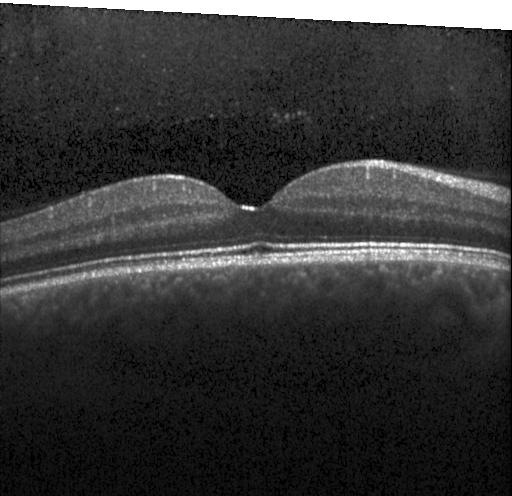

Instrument: Heidelberg Spectralis; OCT line scan; SD-OCT; through the macula — Macular OCT: neither choroidal neovascularization, diabetic macular edema, nor drusen.